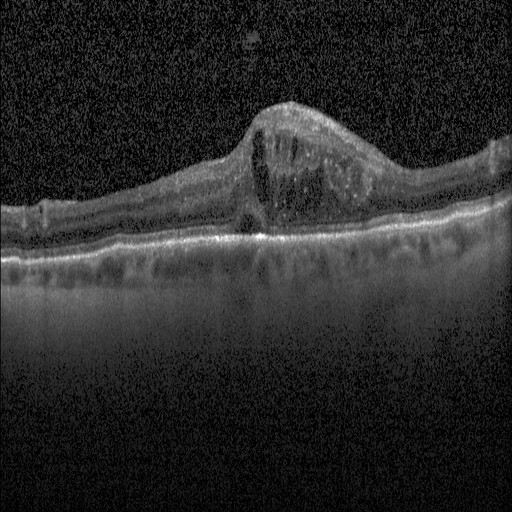 This B-scan demonstrates diabetic macular edema.